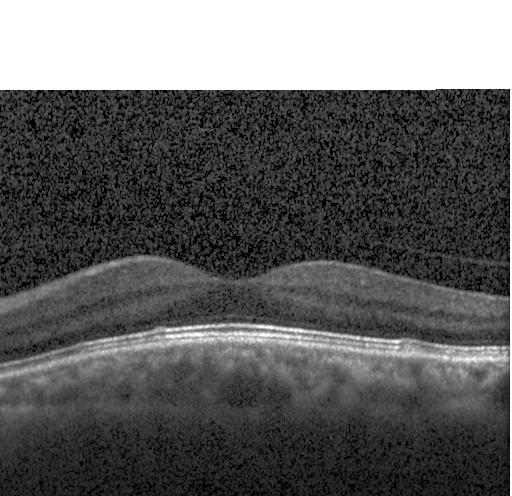

The scan shows no evidence of CNV, DME, or drusen.